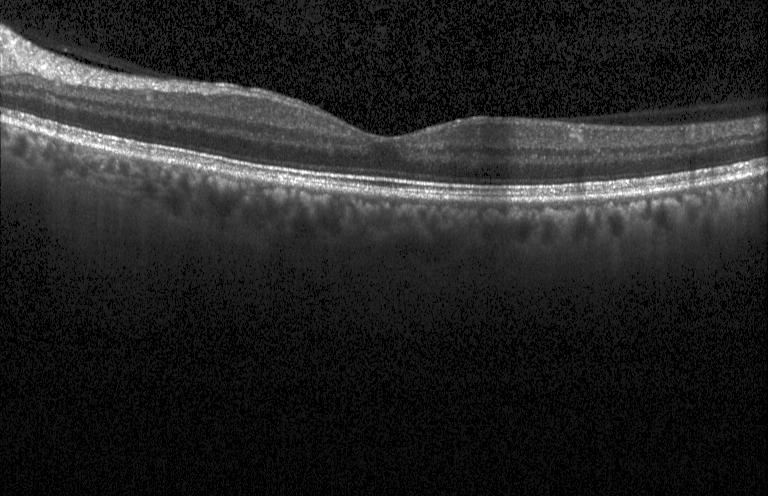

Spectral-domain OCT, fovea-centered, OCT line scan, Heidelberg Spectralis OCT system.
Impression: no choroidal neovascularization, no diabetic macular edema, and no drusen.